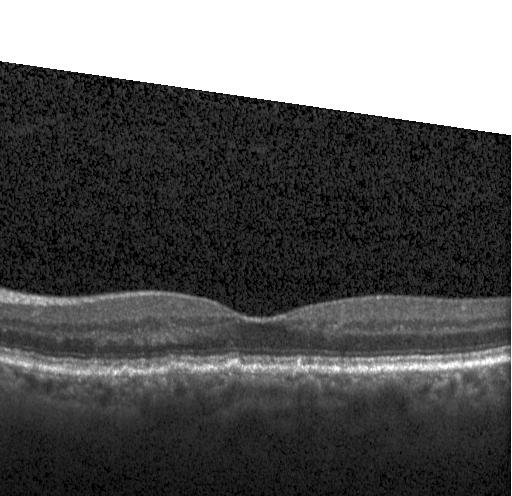 Instrument: Heidelberg Spectralis; retinal OCT B-scan; centered on the fovea — Impression: sub-RPE drusenoid deposits.